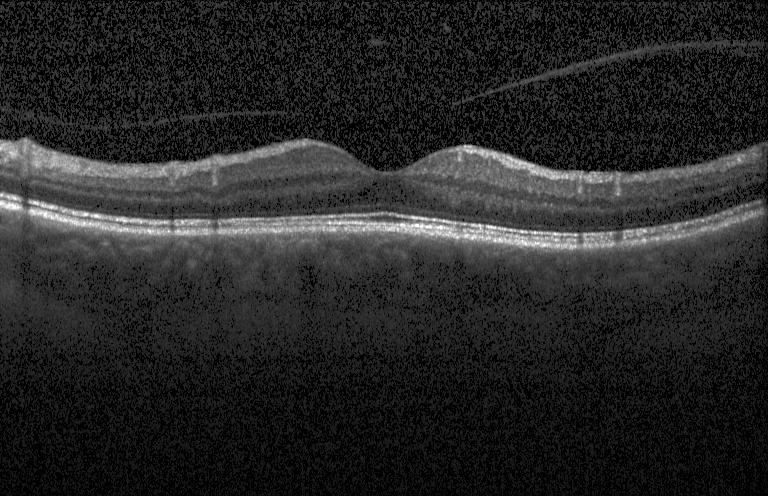 OCT B-scan; spectral-domain optical coherence tomography; instrument: Heidelberg Spectralis; through the macula
Impression: no evidence of choroidal neovascularization, diabetic macular edema, or drusen.